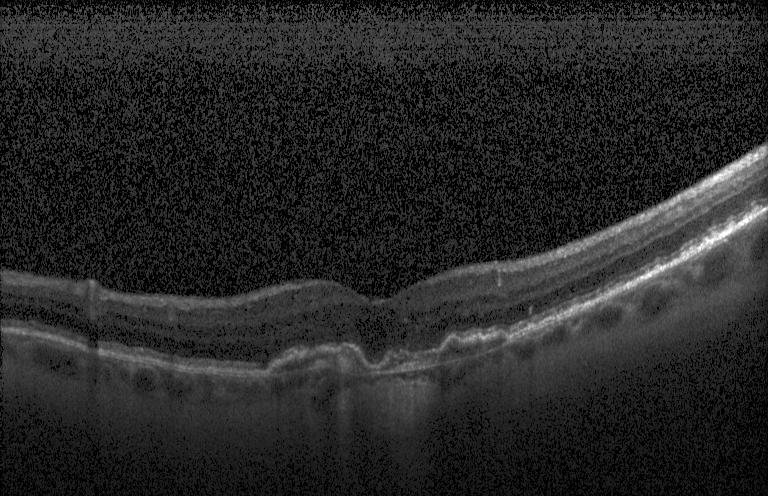

OCT scan showing a choroidal neovascular membrane.